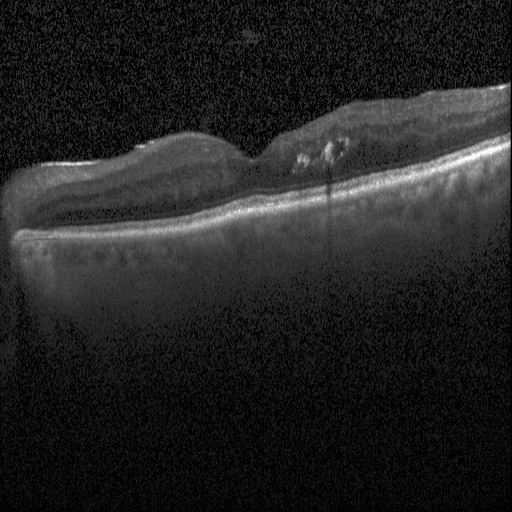

Finding: diabetic macular edema (DME).